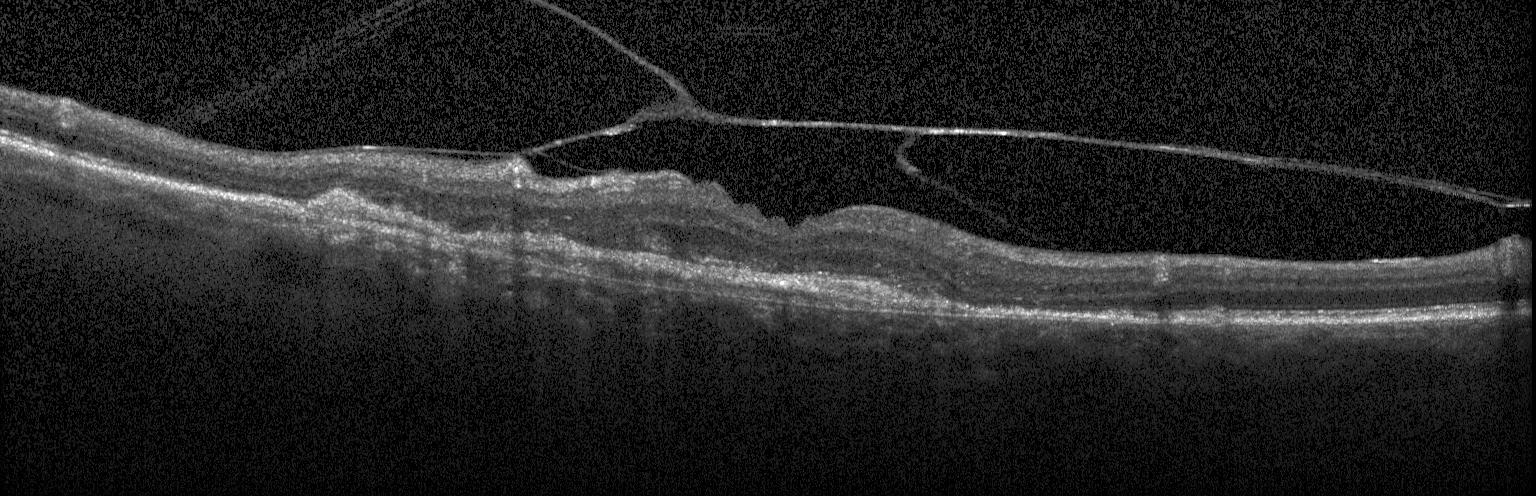

Optical coherence tomography B-scan; fovea-centered; instrument: Heidelberg Spectralis; spectral-domain optical coherence tomography
Finding: choroidal neovascularization.